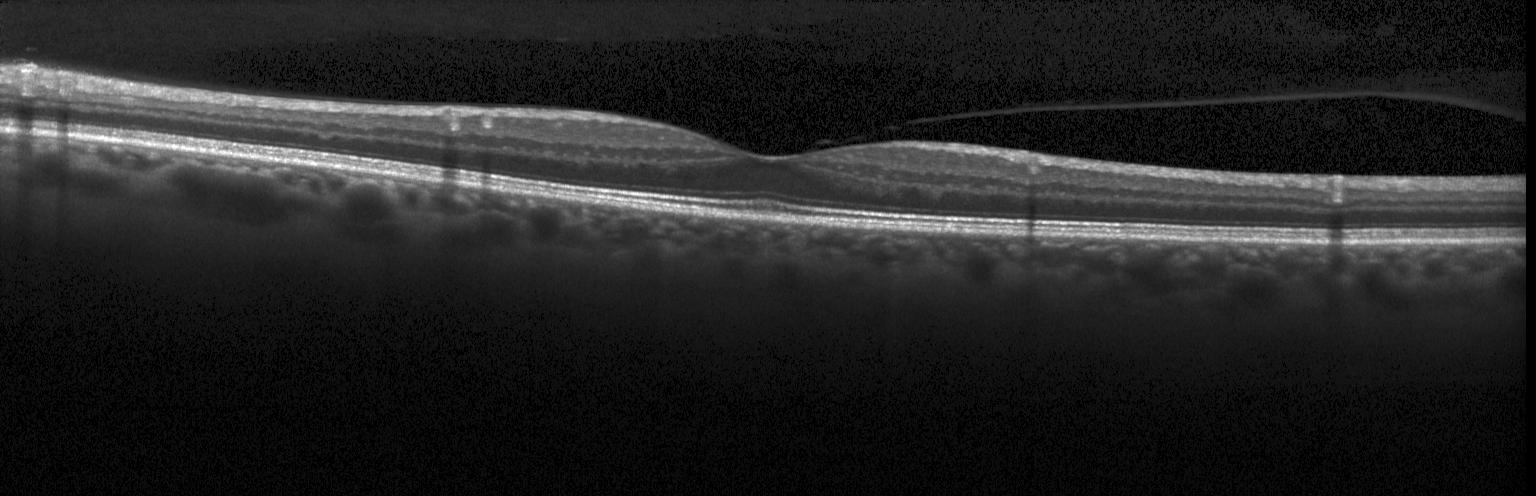

Impression: no evidence of choroidal neovascularization, diabetic macular edema, or drusen.